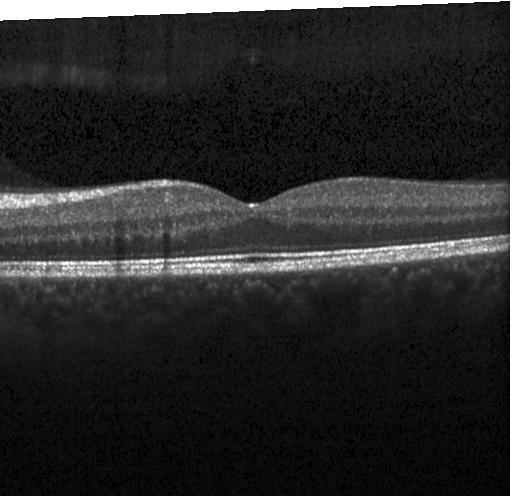 Macular OCT: no evidence of choroidal neovascularization, diabetic macular edema, or drusen.